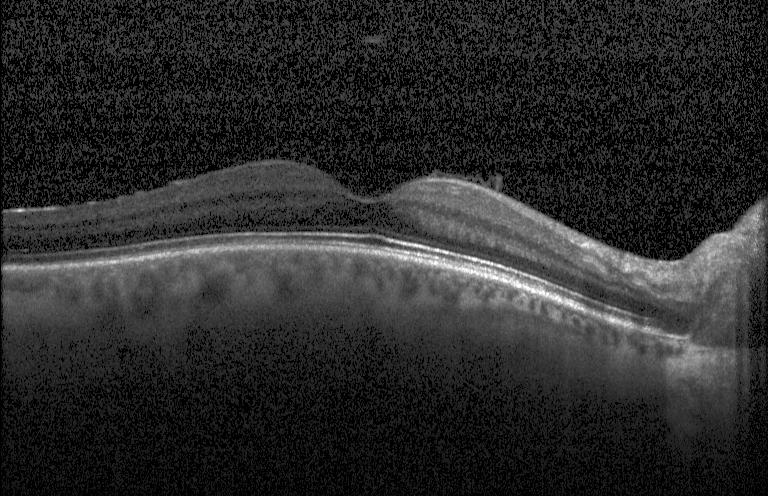 OCT finding: no evidence of CNV, DME, or drusen.